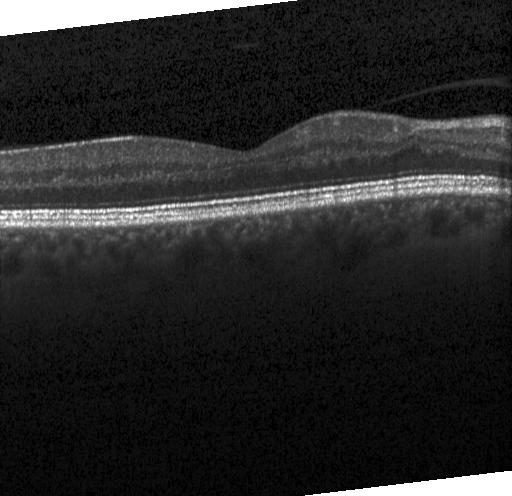

Impression: neither CNV, DME, nor drusen.